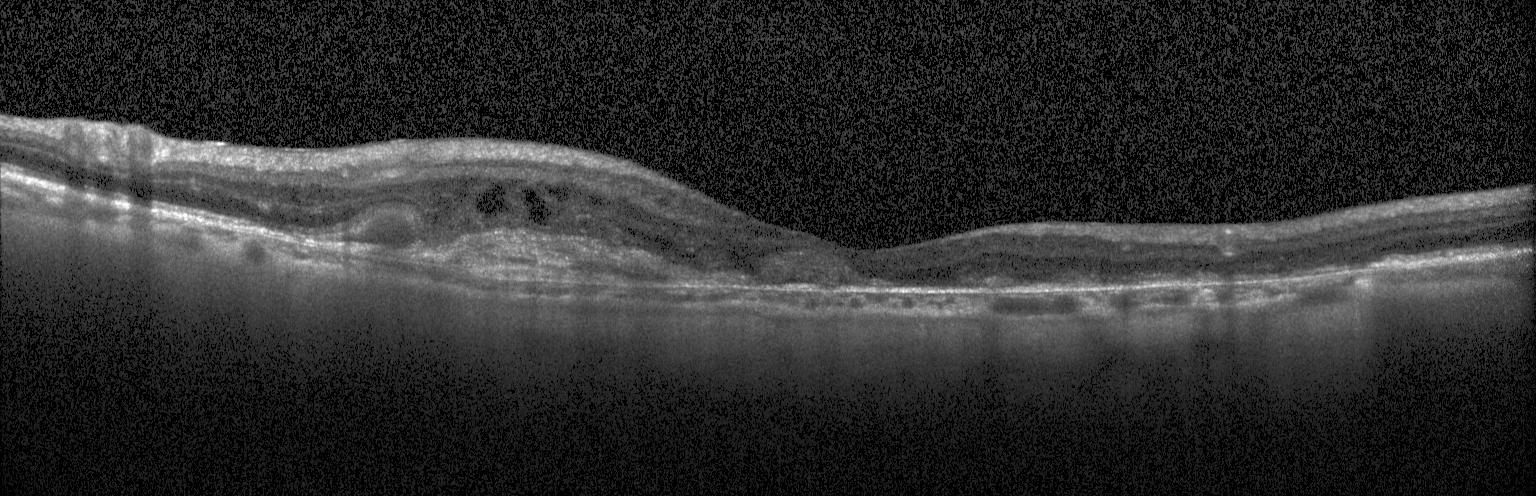 Acquired on a Heidelberg Spectralis. SD-OCT. Fovea-centered. OCT B-scan. Dx: choroidal neovascularization (CNV).